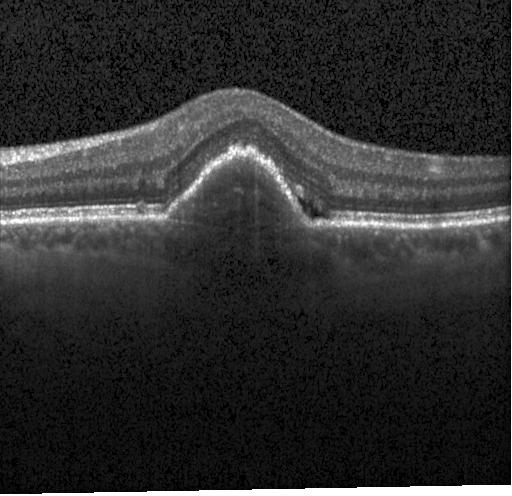 Retinal OCT cross-section; fovea-centered; spectral-domain optical coherence tomography; acquired on a Heidelberg Spectralis
Diagnosis: choroidal neovascularization.